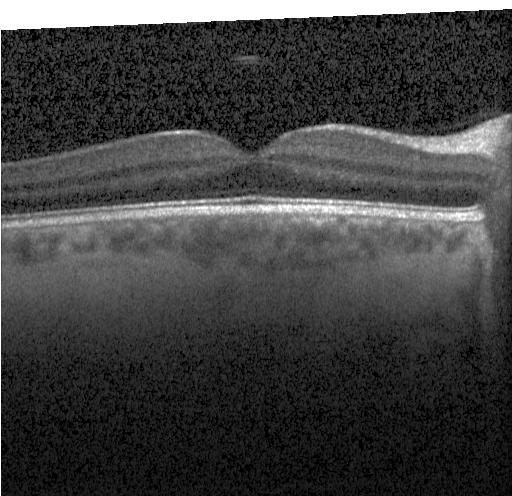
Optical coherence tomography B-scan. Instrument: Heidelberg Spectralis. Finding: neither CNV, DME, nor drusen.